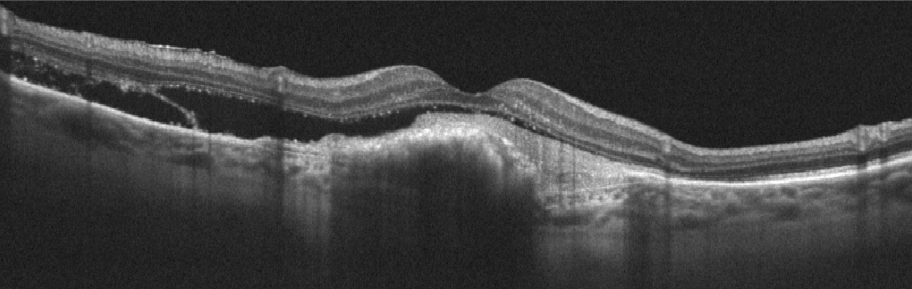

Retinal OCT cross-section. Impression: age-related macular degeneration.